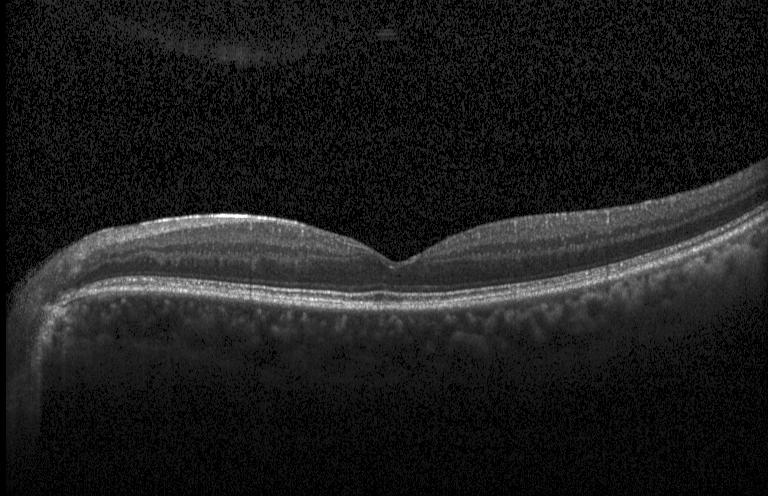 Retinal OCT B-scan.
Diagnosis: no evidence of choroidal neovascularization, diabetic macular edema, or drusen.